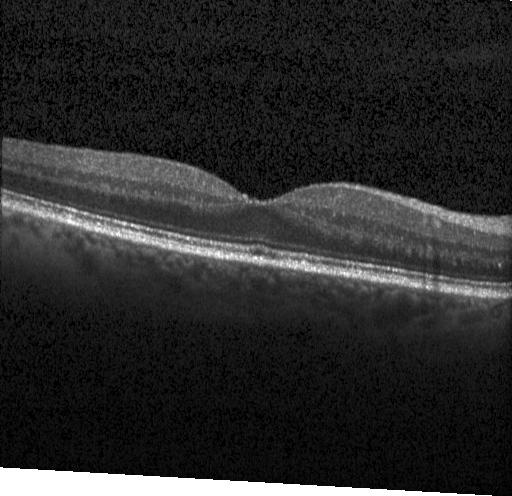
Optical coherence tomography B-scan. Spectral-domain optical coherence tomography. Assessment: no choroidal neovascularization, no diabetic macular edema, and no drusen.